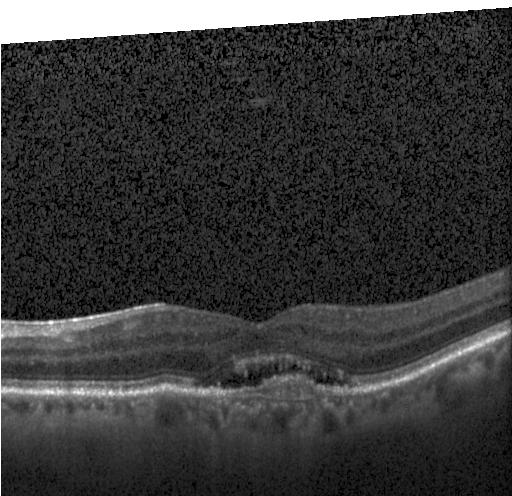

Through the macula, OCT B-scan, spectral-domain OCT
Impression: a choroidal neovascular membrane.